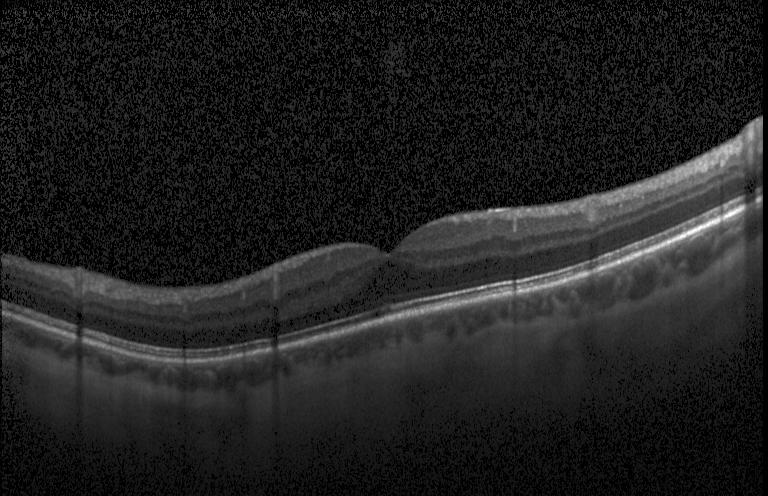
OCT B-scan showing no choroidal neovascularization, no diabetic macular edema, and no drusen.